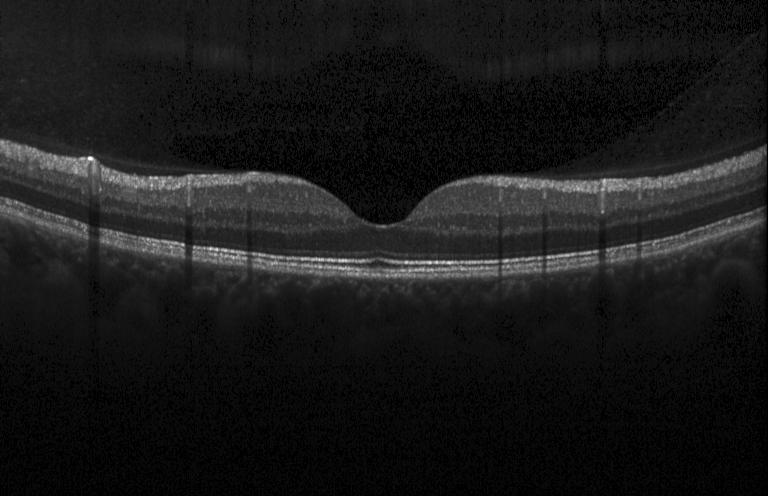
Instrument: Heidelberg Spectralis · optical coherence tomography B-scan — Finding: no choroidal neovascularization, no diabetic macular edema, and no drusen.